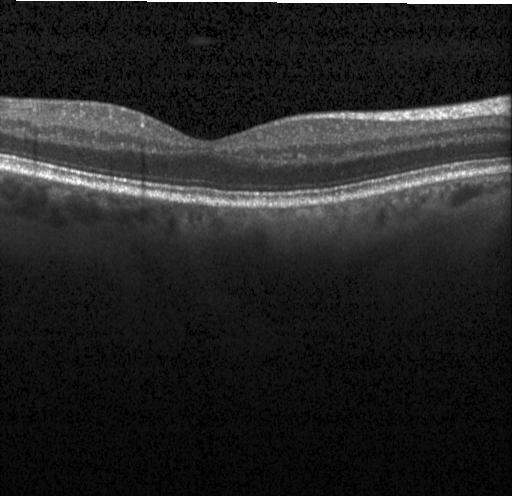

Centered on the fovea, instrument: Heidelberg Spectralis, retinal OCT cross-section
This B-scan demonstrates neither CNV, DME, nor drusen.